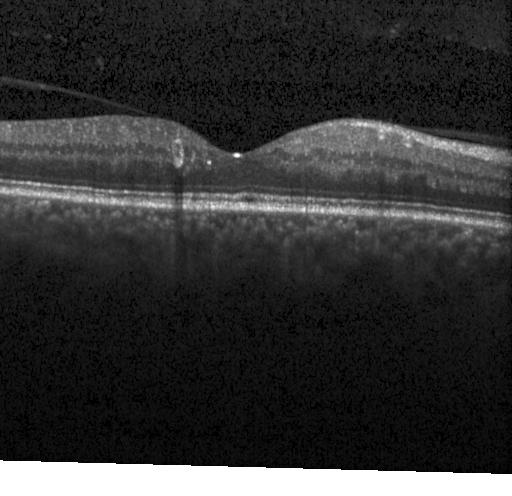

Fovea-centered, retinal OCT B-scan, spectral-domain optical coherence tomography. Finding: no CNV, DME, or drusen.